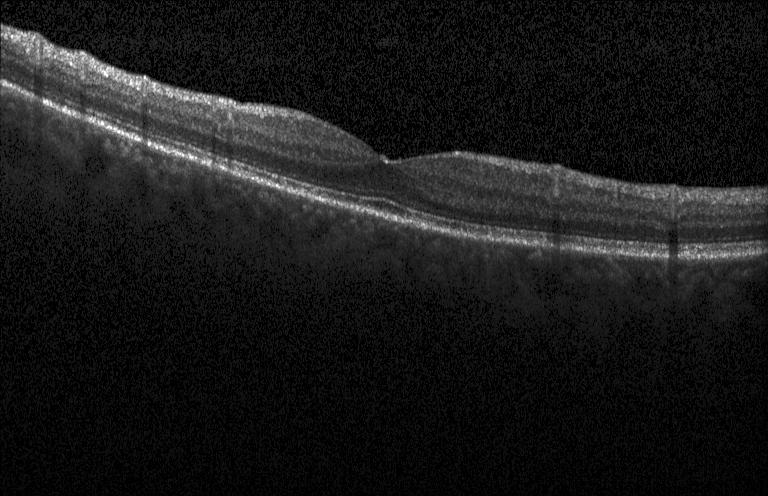
Dx: no choroidal neovascularization, diabetic macular edema, or drusen.